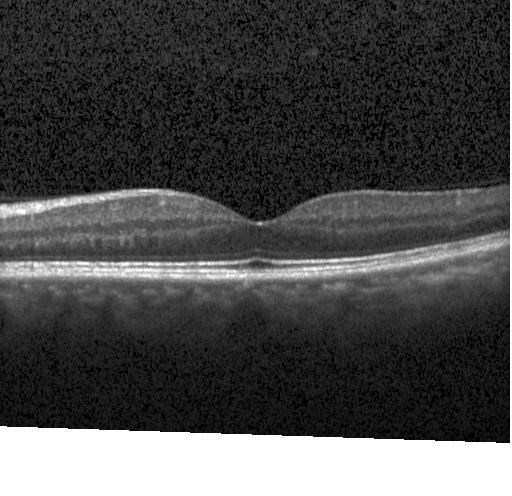 Spectral-domain OCT, retinal OCT cross-section
The scan shows no choroidal neovascularization, diabetic macular edema, or drusen.